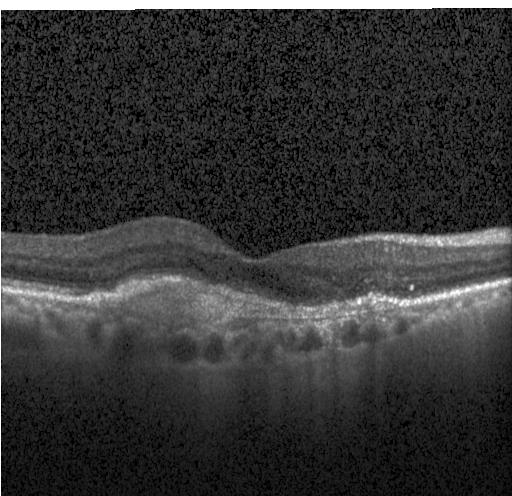 SD-OCT, optical coherence tomography B-scan, Heidelberg Spectralis OCT system, macular scan
OCT finding: CNV.